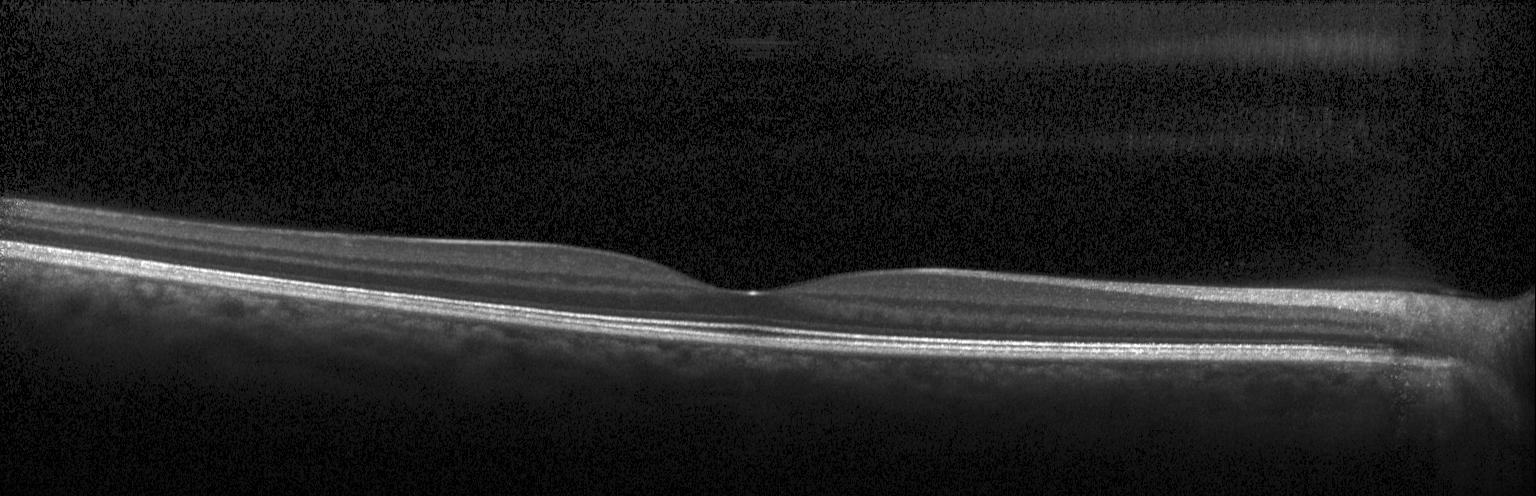

Finding: no evidence of CNV, DME, or drusen.